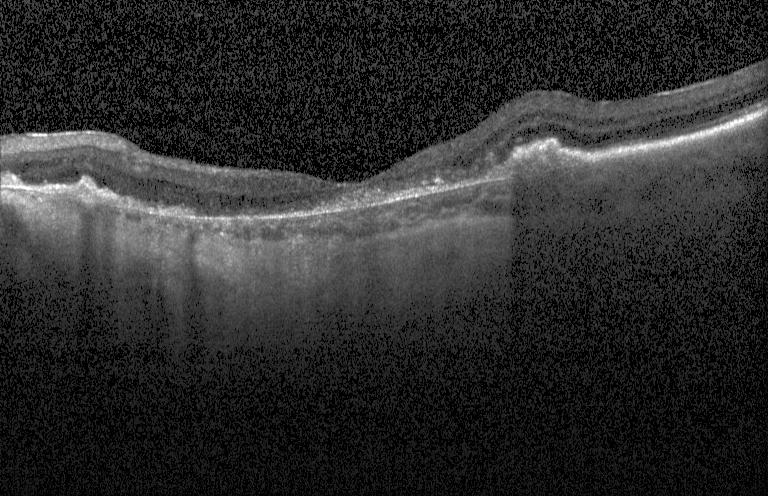
Macular OCT: choroidal neovascularization.